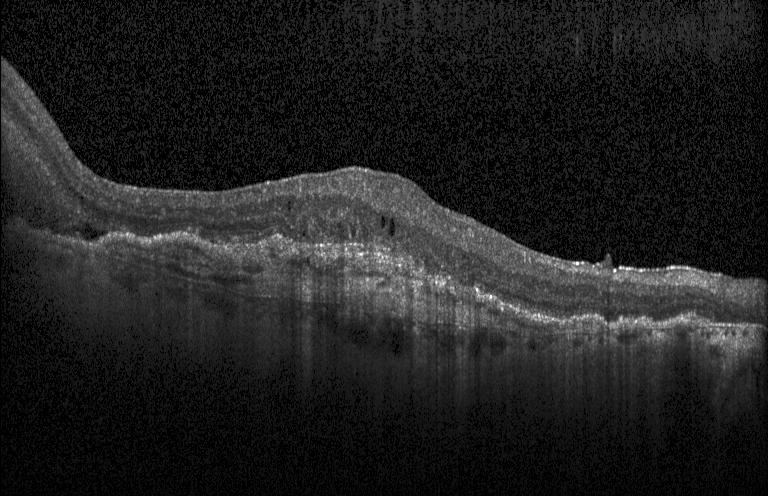
Finding: choroidal neovascularization.